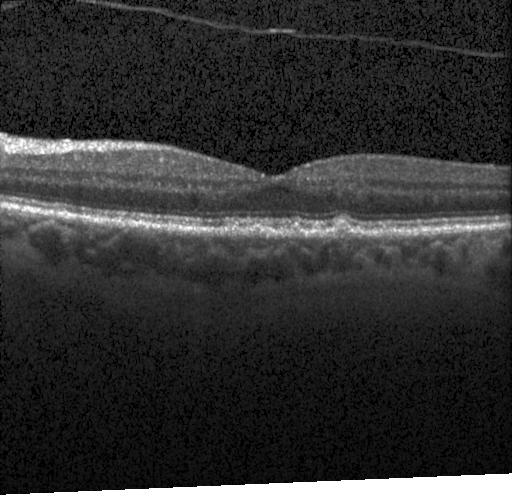
Fovea-centered; optical coherence tomography B-scan — Dx: drusen.